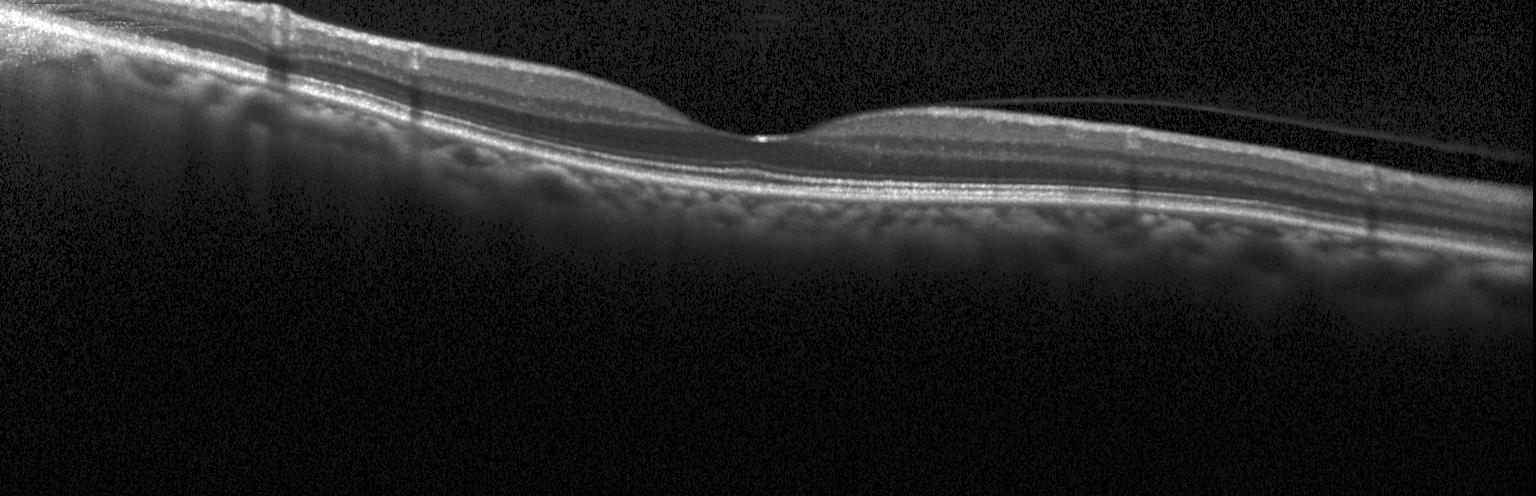
Retinal OCT cross-section showing no evidence of choroidal neovascularization, diabetic macular edema, or drusen.